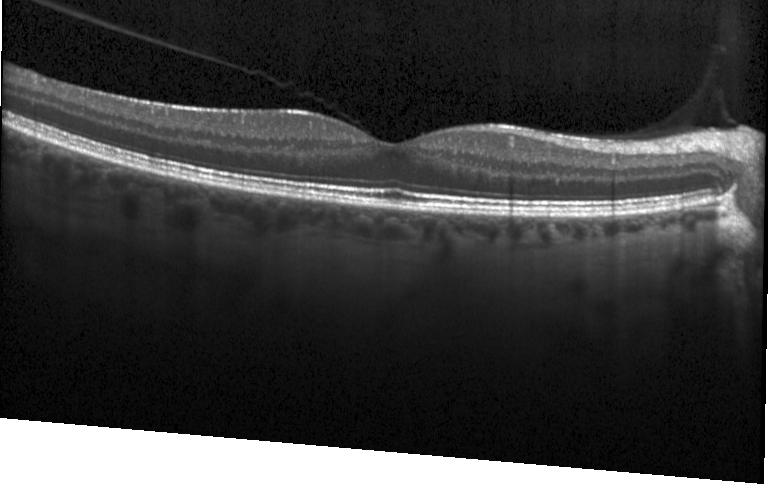 No choroidal neovascularization, diabetic macular edema, or drusen.